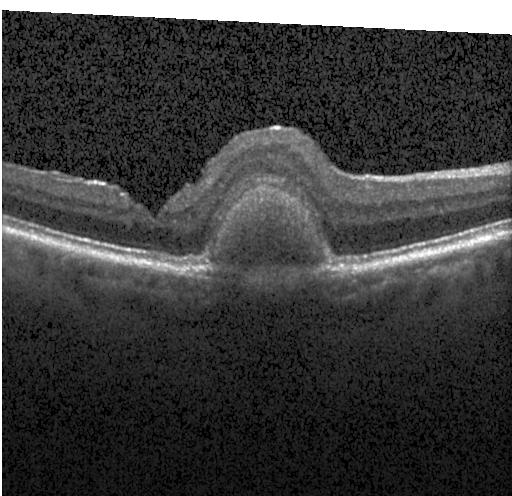

Spectral-domain OCT, acquired on a Heidelberg Spectralis, OCT line scan, through the macula. Diagnosis: a choroidal neovascular membrane.